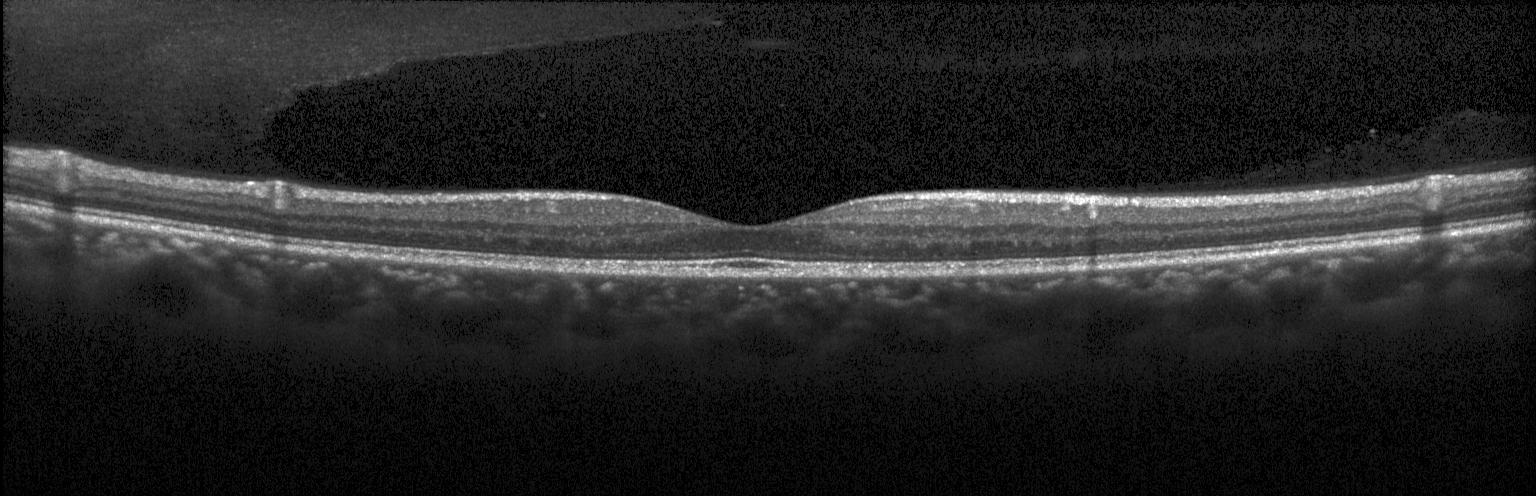
OCT B-scan — Finding: no CNV, no DME, and no drusen.